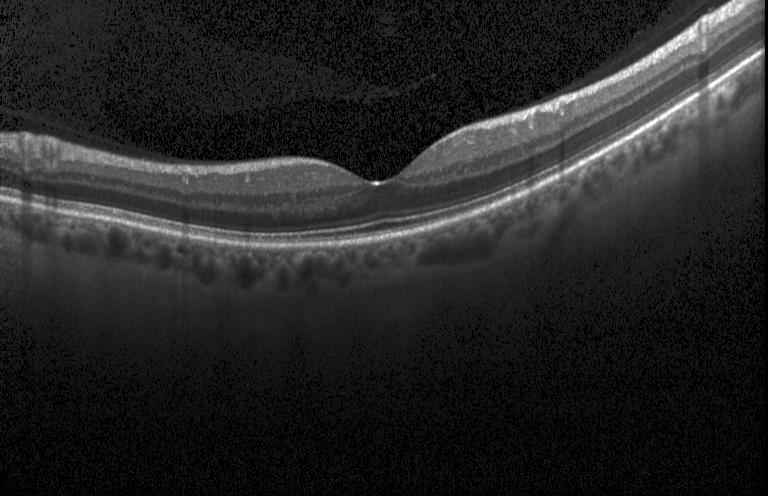

Diagnosis: no evidence of choroidal neovascularization, diabetic macular edema, or drusen.